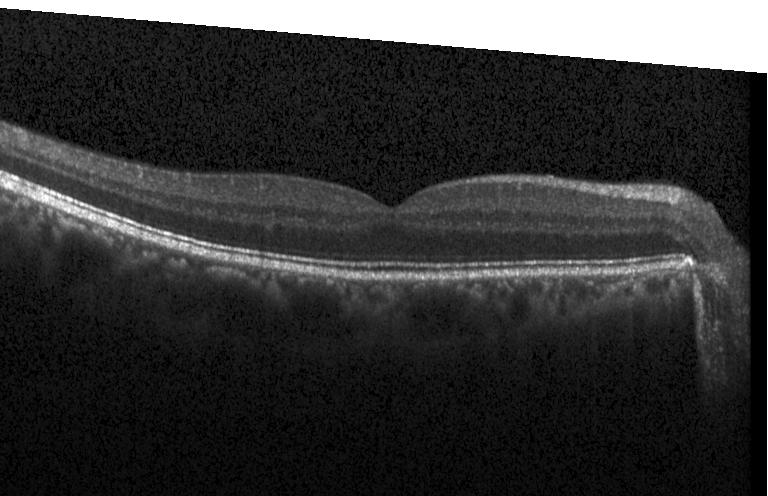
OCT finding: no evidence of choroidal neovascularization, diabetic macular edema, or drusen.